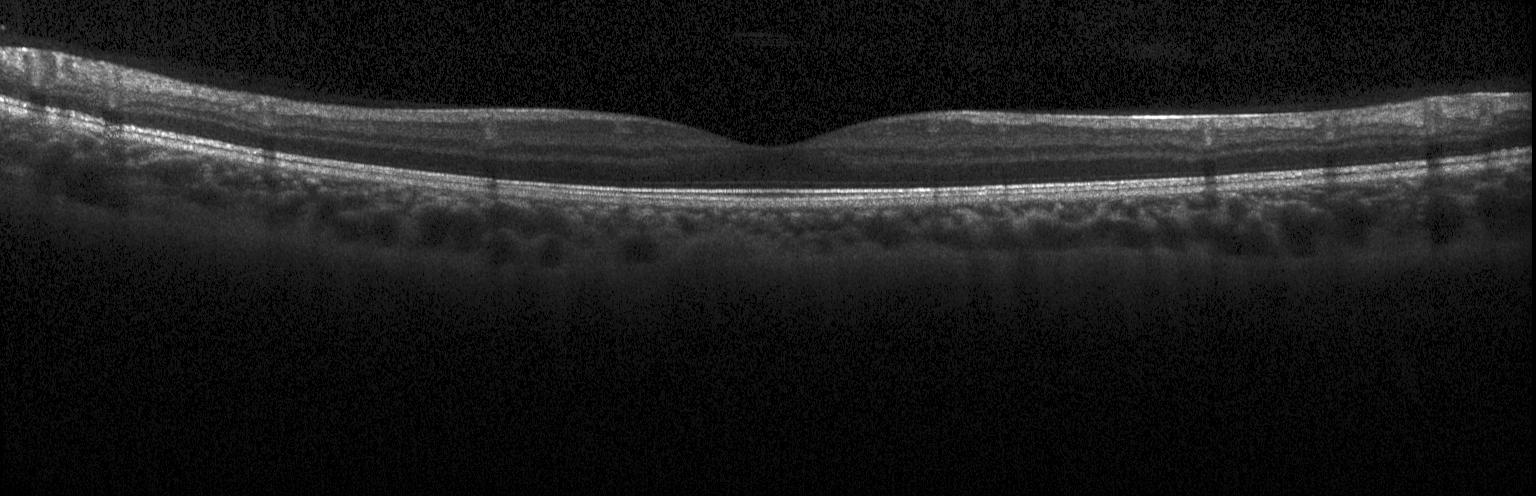
Macular scan · OCT B-scan.
Impression: no choroidal neovascularization, no diabetic macular edema, and no drusen.